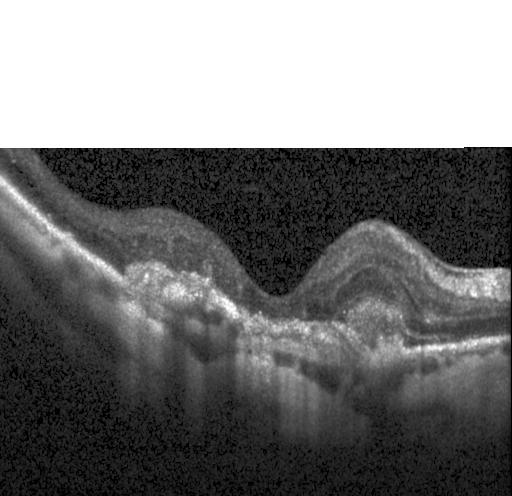
Dx: a choroidal neovascular membrane.